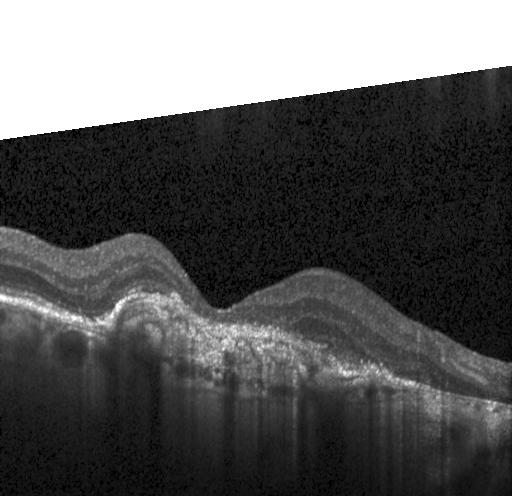

OCT line scan
Assessment: choroidal neovascularization (CNV).